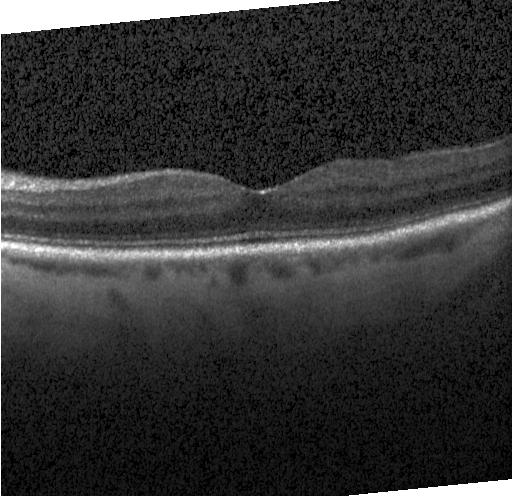

OCT line scan
Assessment: neither choroidal neovascularization, diabetic macular edema, nor drusen.